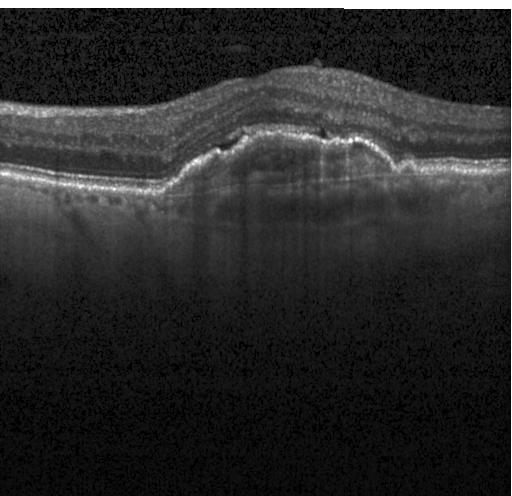

Macular OCT: choroidal neovascularization (CNV).